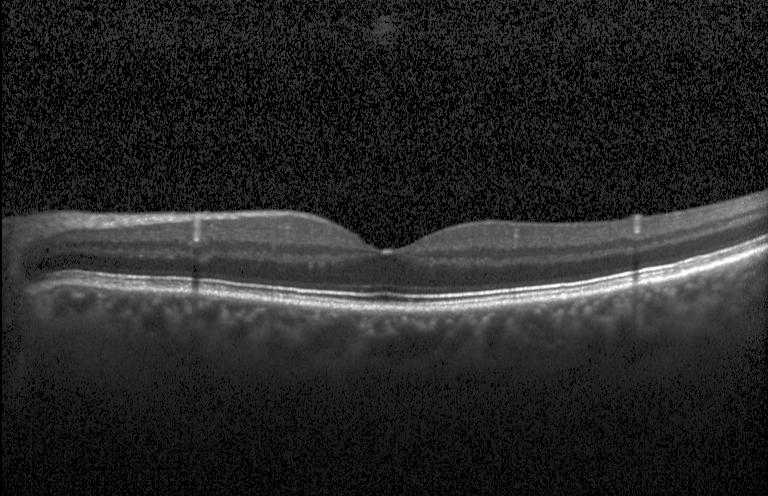 Retinal OCT cross-section — Neither choroidal neovascularization, diabetic macular edema, nor drusen.